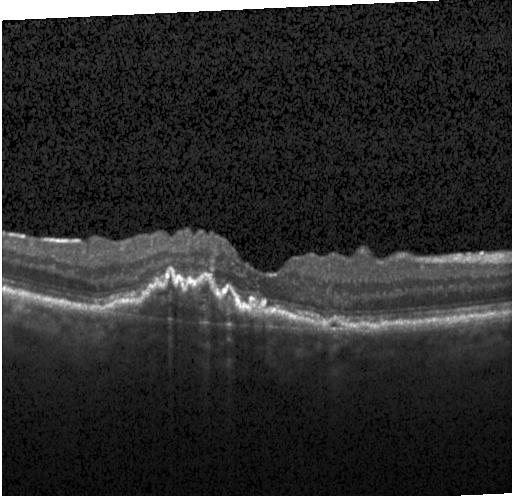 Dx: a choroidal neovascular membrane.